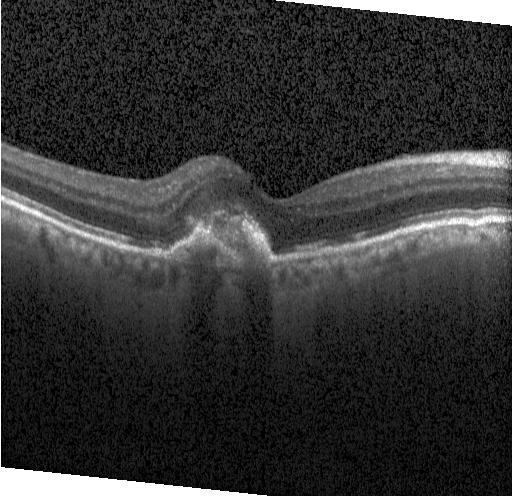 Retinal OCT B-scan, through the macula — Diagnosis: CNV.